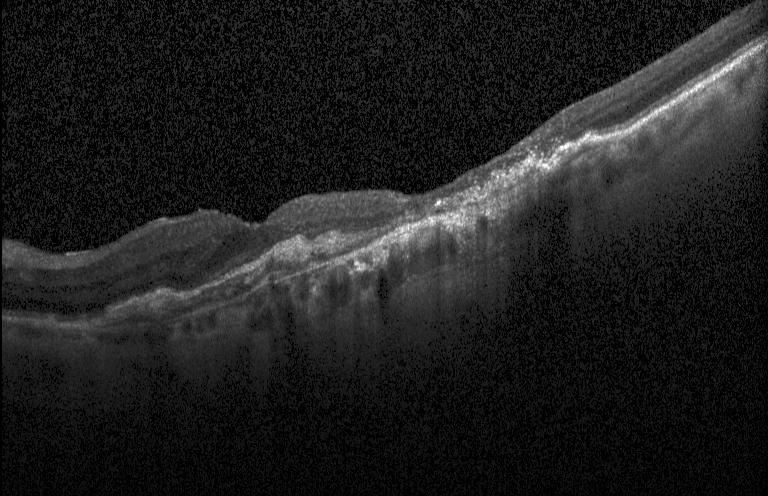

OCT B-scan. Spectral-domain optical coherence tomography — Impression: a choroidal neovascular membrane.